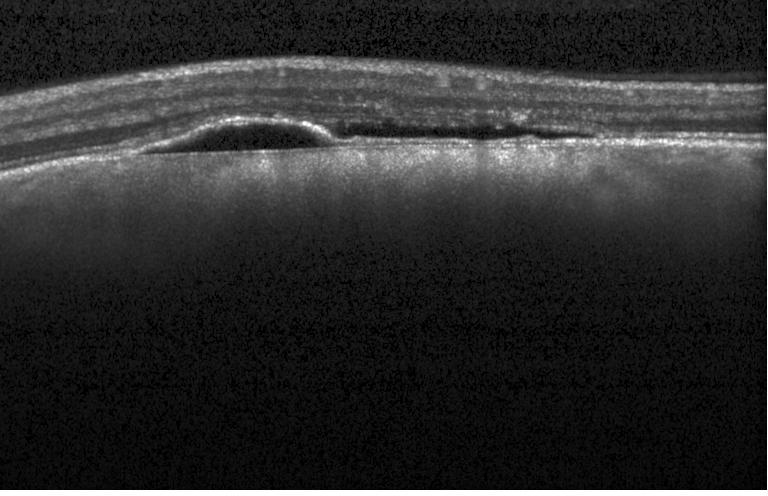 Macular OCT demonstrating a choroidal neovascular membrane.